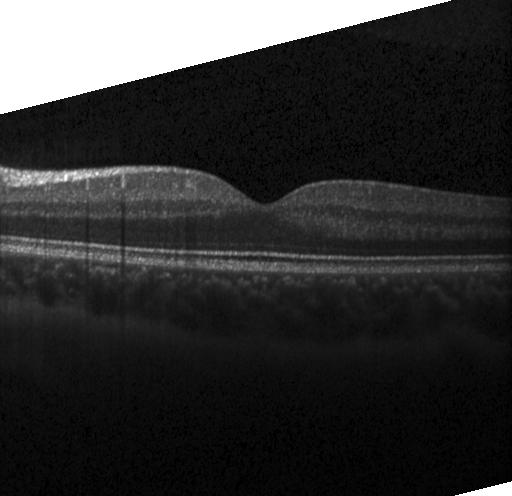

Heidelberg Spectralis OCT system · through the macula · spectral-domain OCT · OCT B-scan
Impression: no choroidal neovascularization, diabetic macular edema, or drusen.